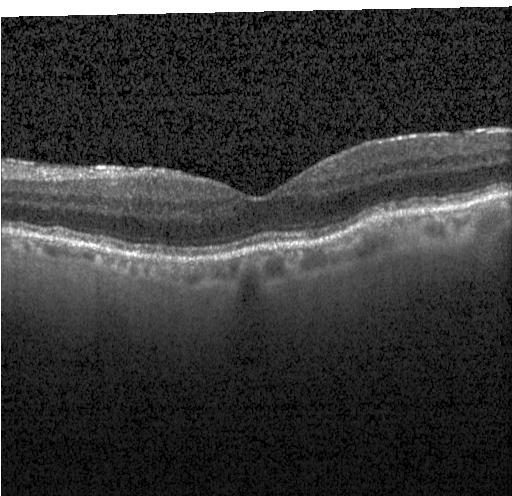

OCT B-scan — Finding: no choroidal neovascularization, no diabetic macular edema, and no drusen.